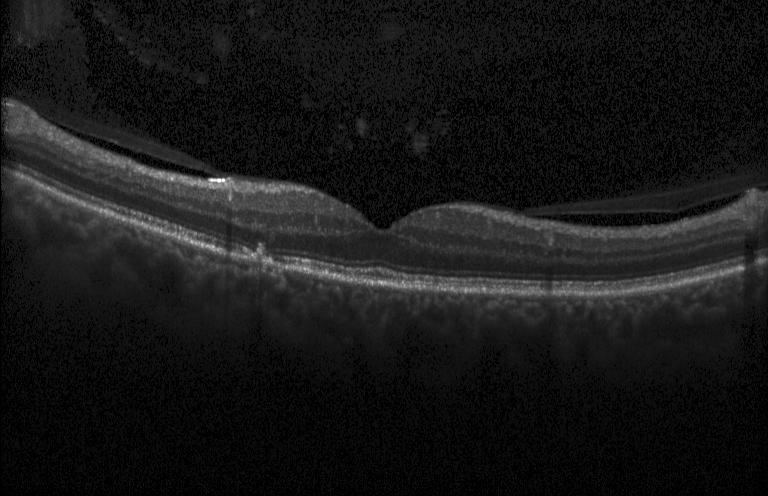

Optical coherence tomography scan — Diagnosis: multiple drusen.